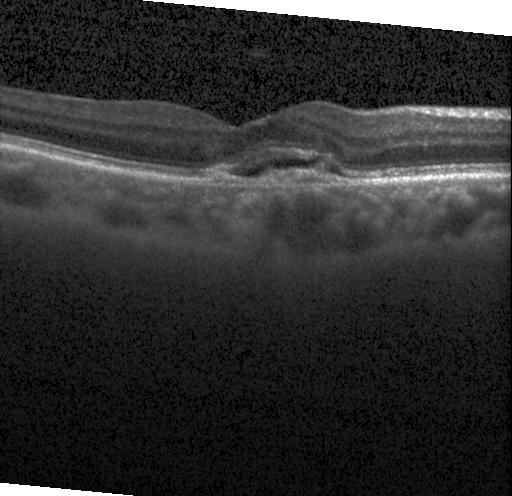 OCT line scan
A choroidal neovascular membrane.